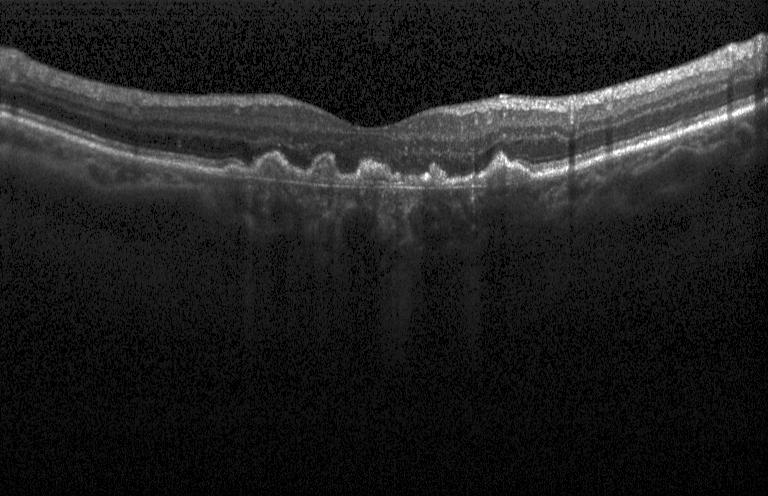
OCT line scan; Heidelberg Spectralis OCT system; spectral-domain optical coherence tomography
Choroidal neovascularization.